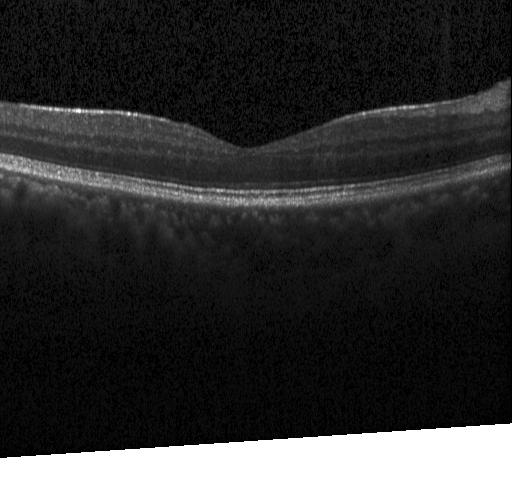 Through the macula, Heidelberg Spectralis, OCT B-scan. Dx: neither choroidal neovascularization, diabetic macular edema, nor drusen.